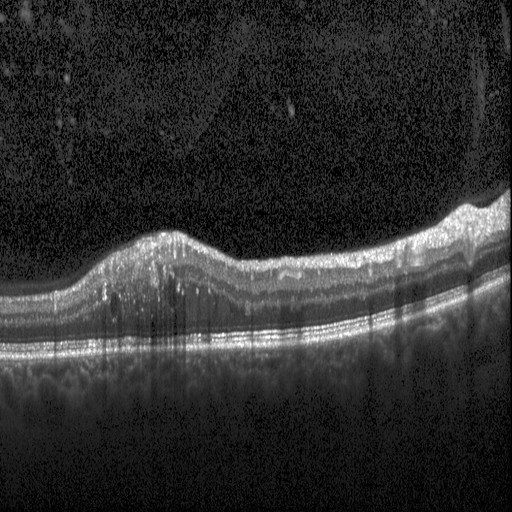
This B-scan demonstrates DME.